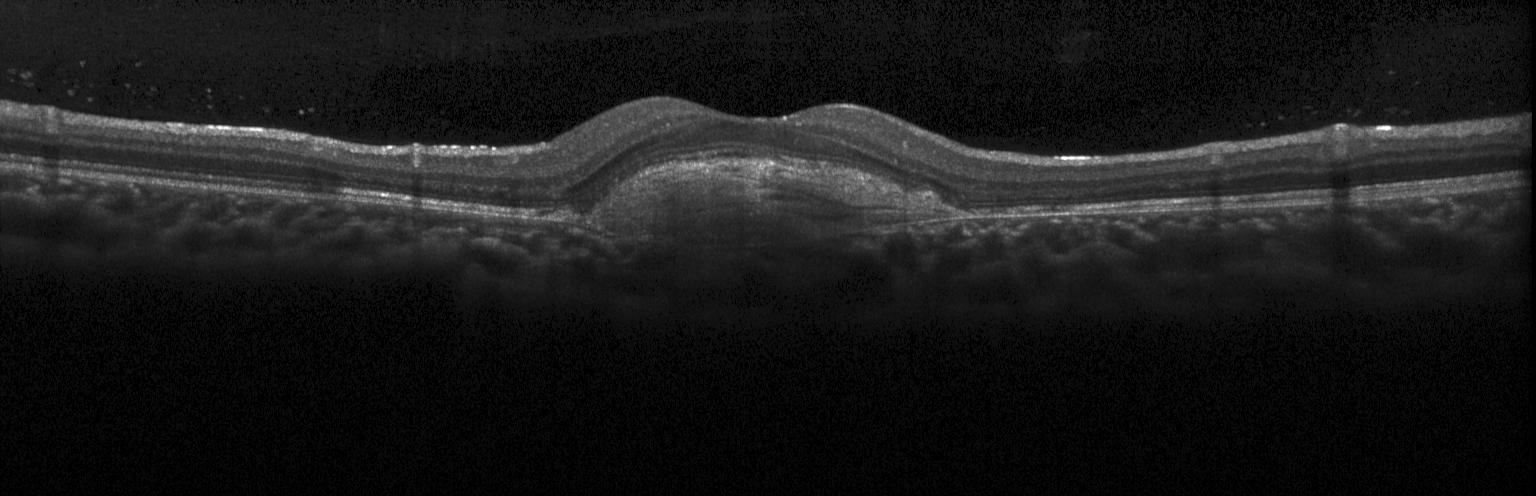 Retinal OCT cross-section — This B-scan demonstrates choroidal neovascularization (CNV).